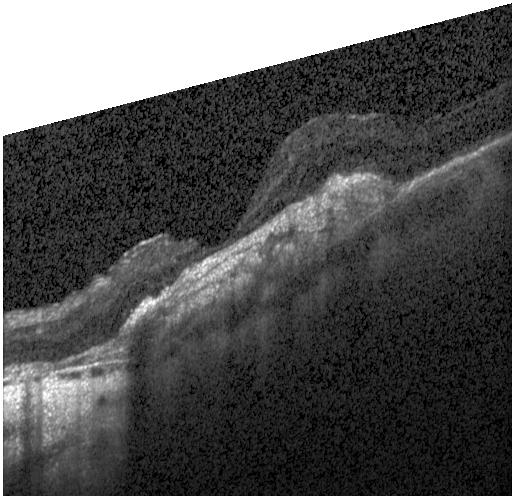

Acquired on a Heidelberg Spectralis; spectral-domain OCT; OCT line scan; horizontal scan through the fovea.
OCT finding: choroidal neovascularization.